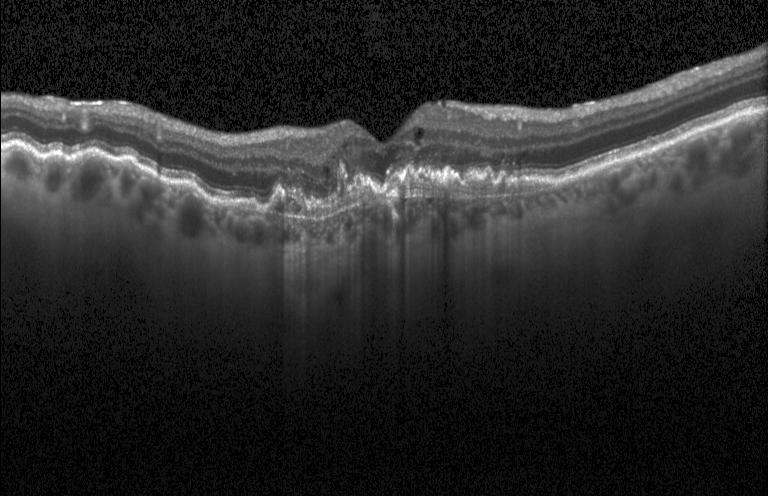
Impression: CNV.